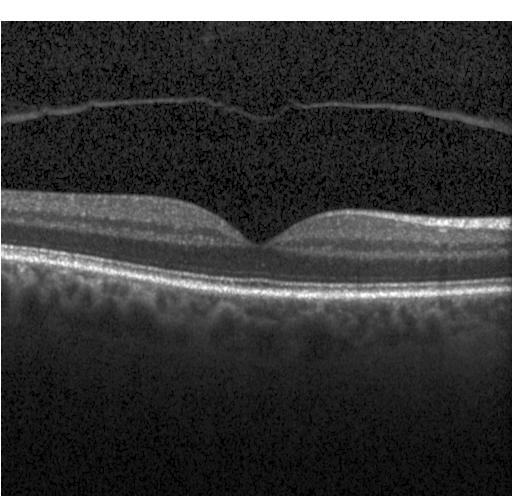

Diagnosis: no choroidal neovascularization, diabetic macular edema, or drusen.